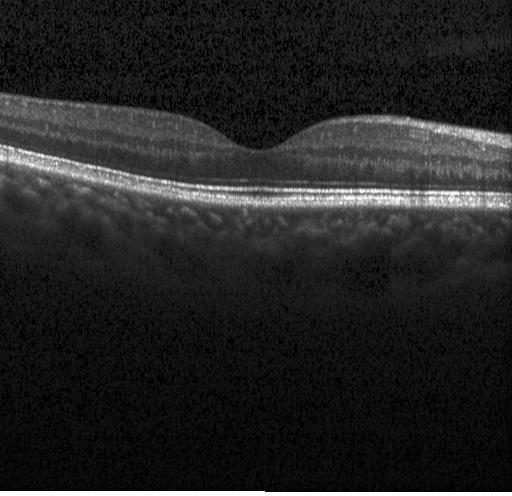
SD-OCT, retinal OCT B-scan, centered on the fovea, instrument: Heidelberg Spectralis. No choroidal neovascularization, diabetic macular edema, or drusen.